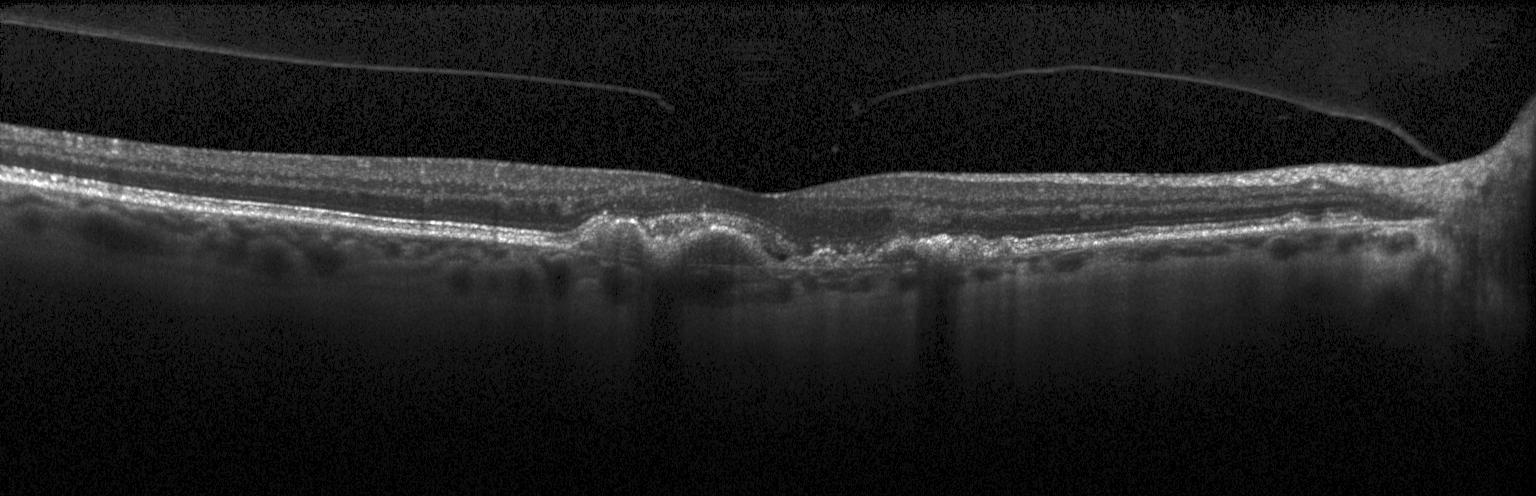 Spectral-domain OCT, horizontal scan through the fovea, retinal OCT B-scan, Heidelberg Spectralis
Impression: choroidal neovascularization.